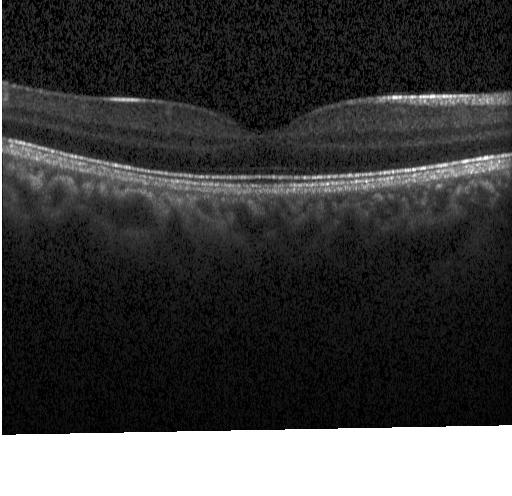

OCT line scan. Macular OCT: no choroidal neovascularization, diabetic macular edema, or drusen.